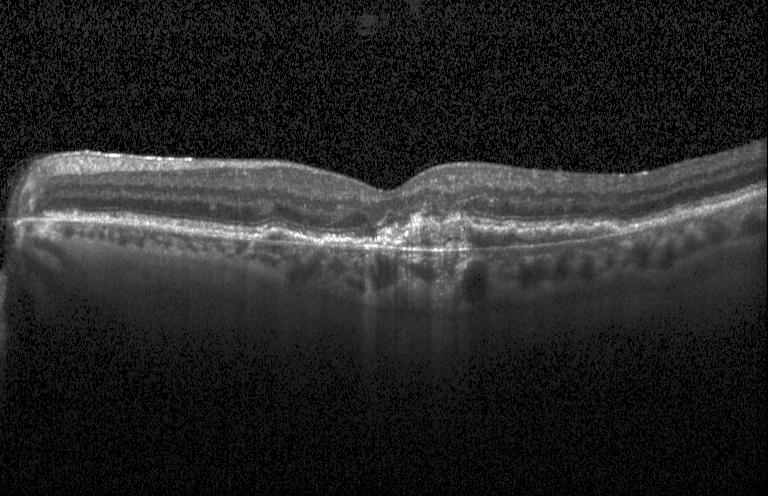 Spectral-domain optical coherence tomography. Optical coherence tomography scan. Instrument: Heidelberg Spectralis.
Assessment: a choroidal neovascular membrane.